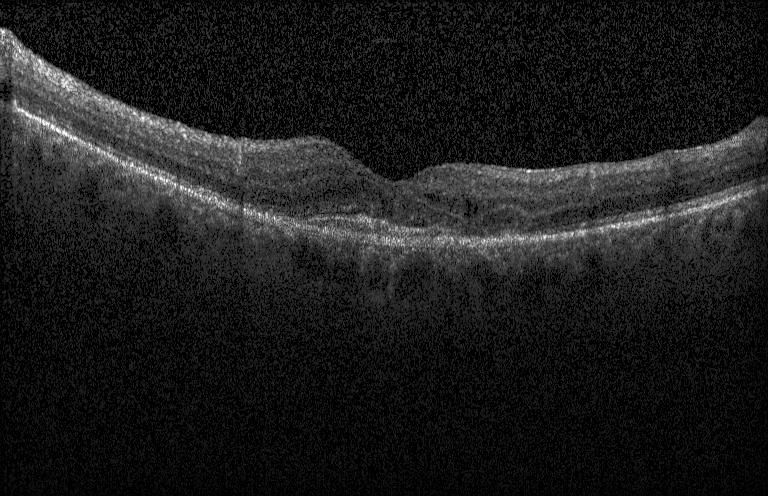

Optical coherence tomography B-scan. OCT finding: CNV.